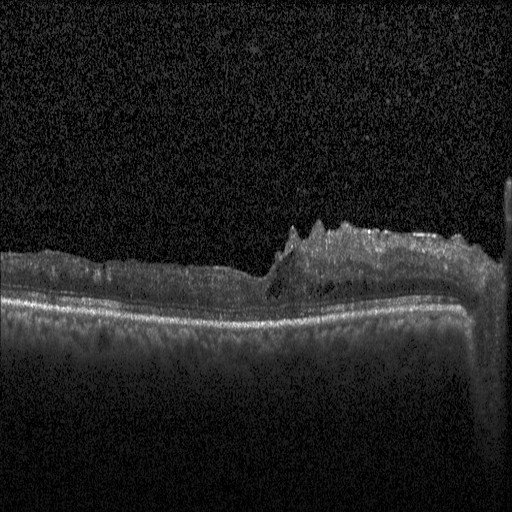 Instrument: Heidelberg Spectralis; spectral-domain OCT; fovea-centered; retinal OCT B-scan.
Dx: diabetic macular edema (DME).